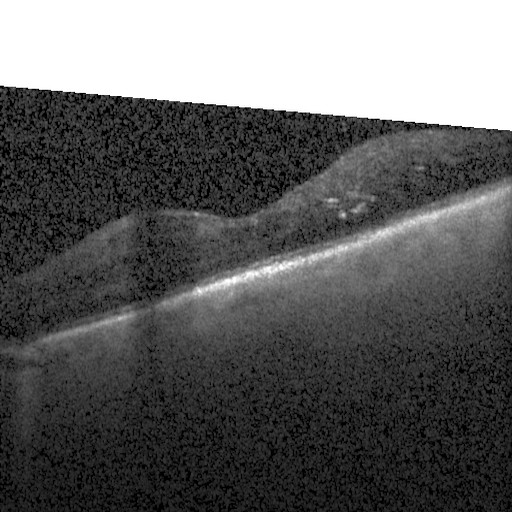
Assessment: diabetic macular edema (DME).